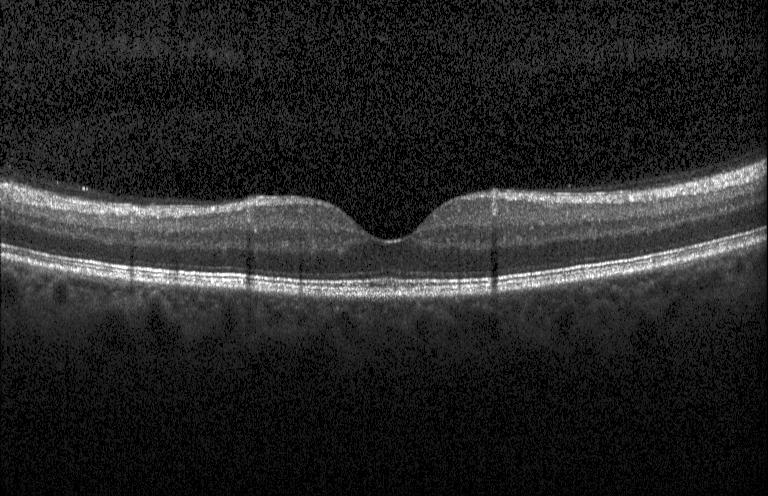
Spectral-domain OCT; OCT line scan — The scan shows no choroidal neovascularization, diabetic macular edema, or drusen.